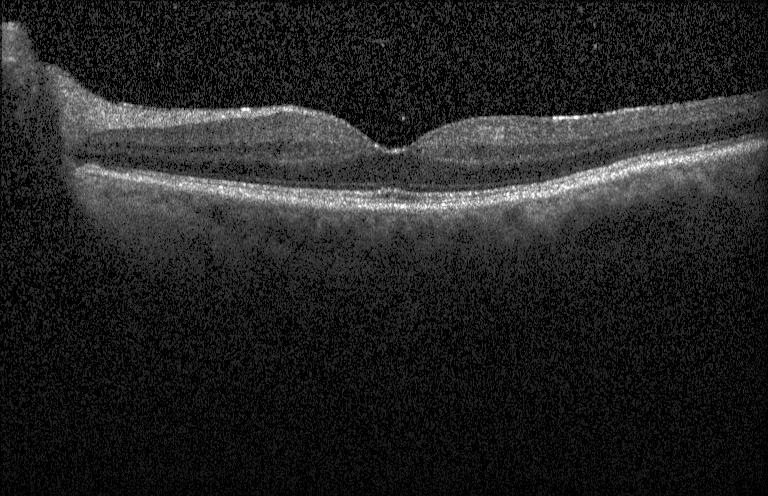 OCT line scan
Impression: neither CNV, DME, nor drusen.